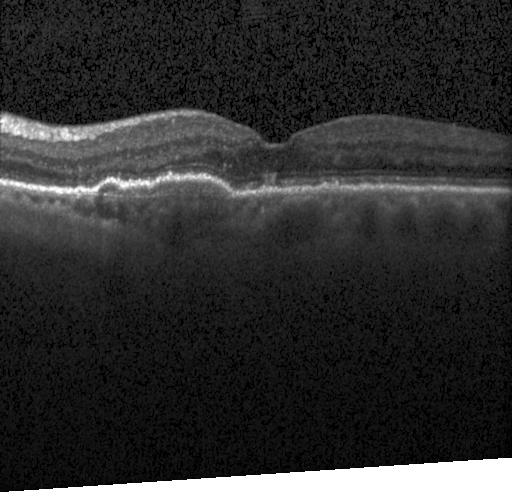
SD-OCT · Heidelberg Spectralis OCT system · OCT B-scan
Macular OCT: a choroidal neovascular membrane.